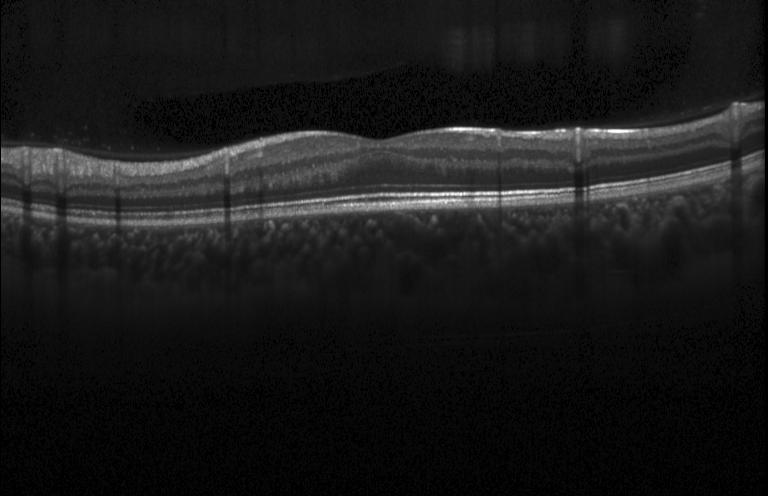 Retinal OCT B-scan
This B-scan demonstrates no evidence of choroidal neovascularization, diabetic macular edema, or drusen.